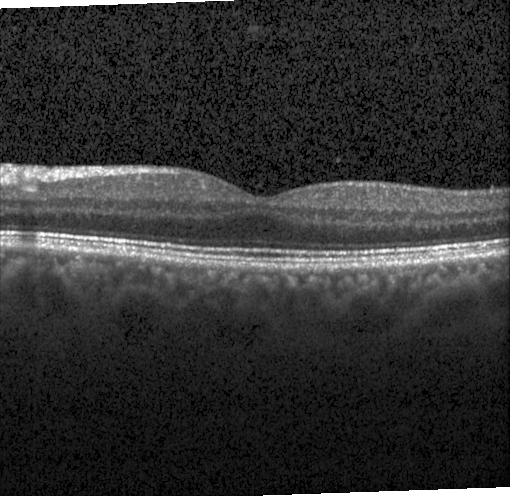
Instrument: Heidelberg Spectralis · optical coherence tomography B-scan
No CNV, no DME, and no drusen.